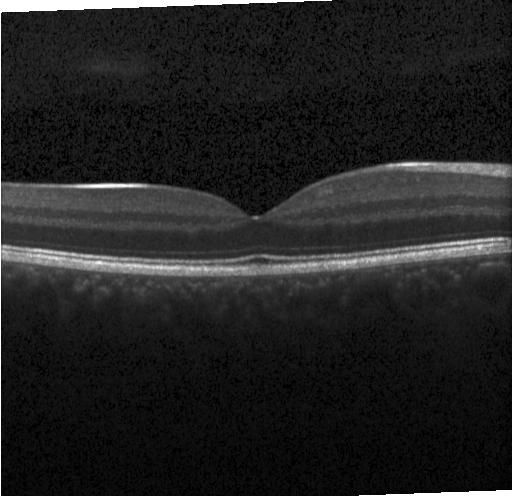

Retinal OCT cross-section showing no CNV, no DME, and no drusen.